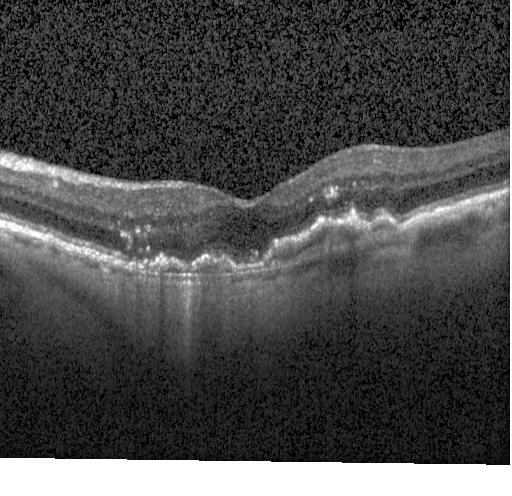
Instrument: Heidelberg Spectralis, optical coherence tomography scan — OCT finding: choroidal neovascularization (CNV).